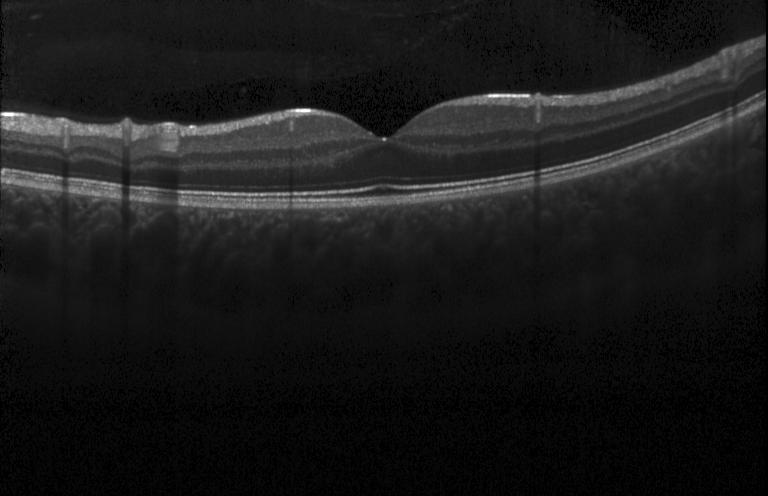 Optical coherence tomography scan · fovea-centered · Heidelberg Spectralis OCT system — Impression: neither choroidal neovascularization, diabetic macular edema, nor drusen.